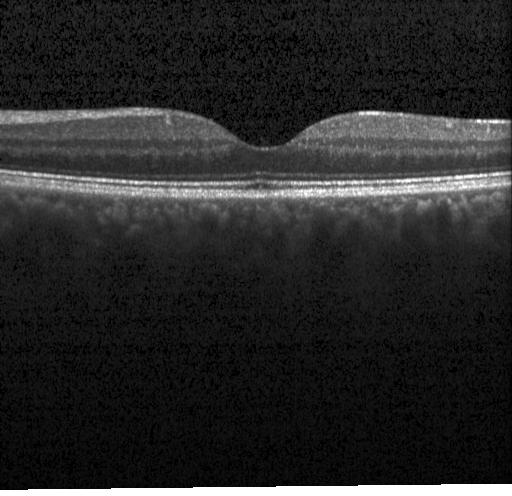 OCT scan showing neither choroidal neovascularization, diabetic macular edema, nor drusen.